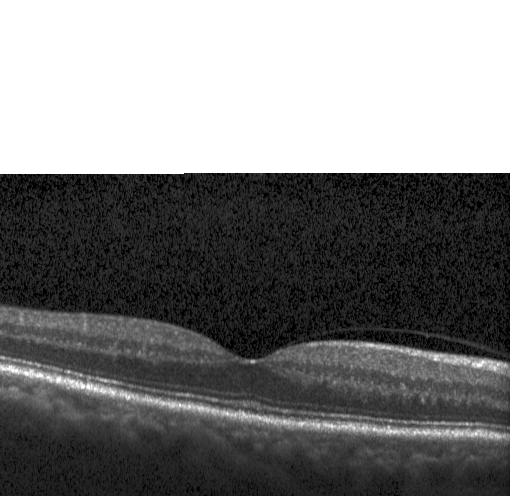
Heidelberg Spectralis, retinal OCT B-scan, horizontal scan through the fovea, spectral-domain OCT
No choroidal neovascularization, no diabetic macular edema, and no drusen.